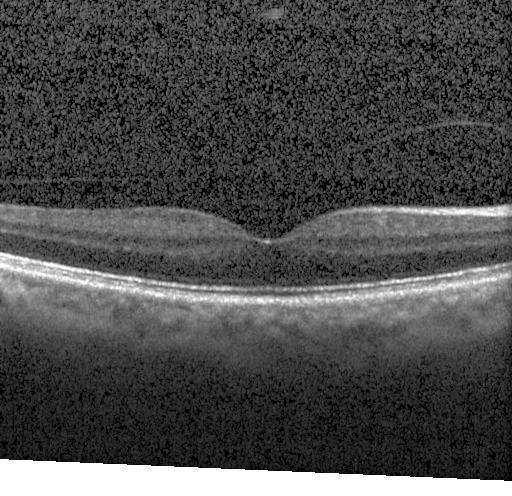

SD-OCT, retinal OCT cross-section — Diagnosis: no evidence of choroidal neovascularization, diabetic macular edema, or drusen.